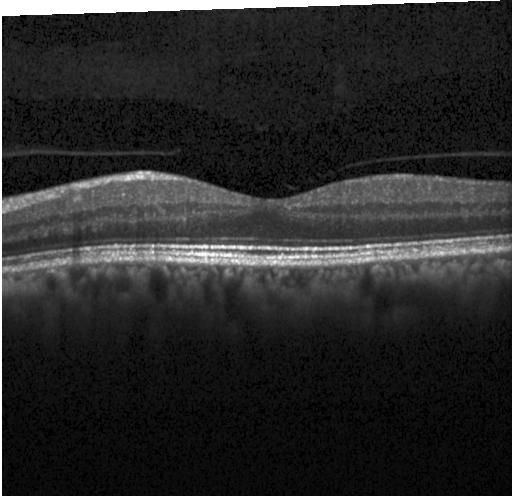
Retinal OCT cross-section showing neither choroidal neovascularization, diabetic macular edema, nor drusen.